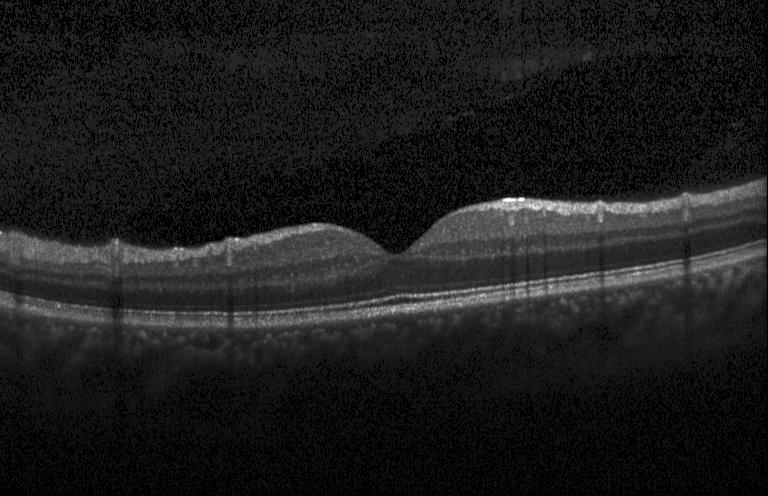

OCT scan showing no evidence of choroidal neovascularization, diabetic macular edema, or drusen.